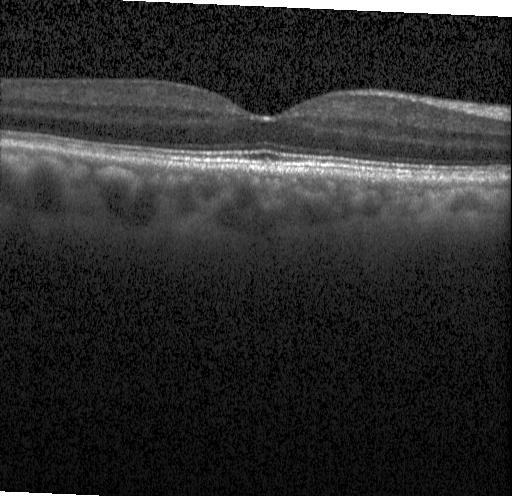

OCT scan showing no evidence of CNV, DME, or drusen.